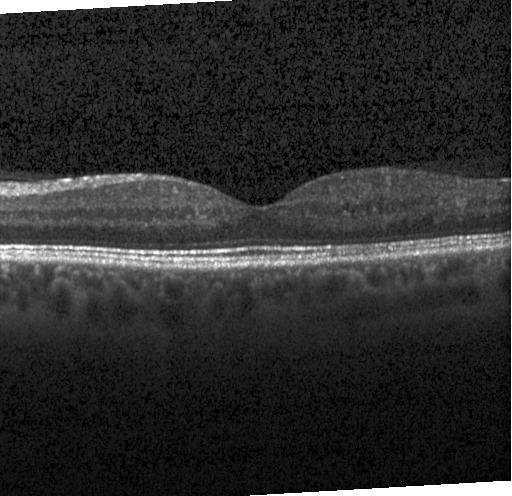

Finding: no choroidal neovascularization, no diabetic macular edema, and no drusen.